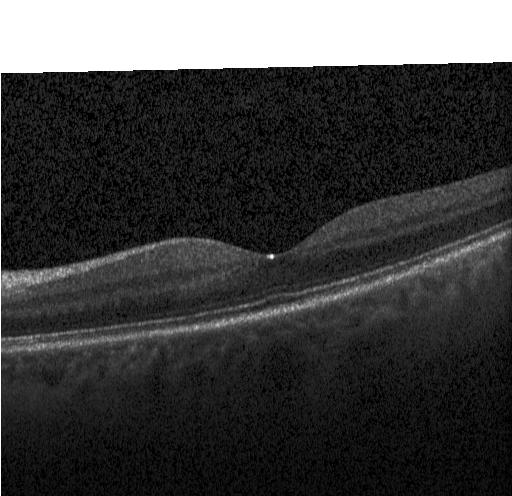
OCT B-scan; spectral-domain optical coherence tomography; acquired on a Heidelberg Spectralis; fovea-centered.
Finding: no choroidal neovascularization, no diabetic macular edema, and no drusen.